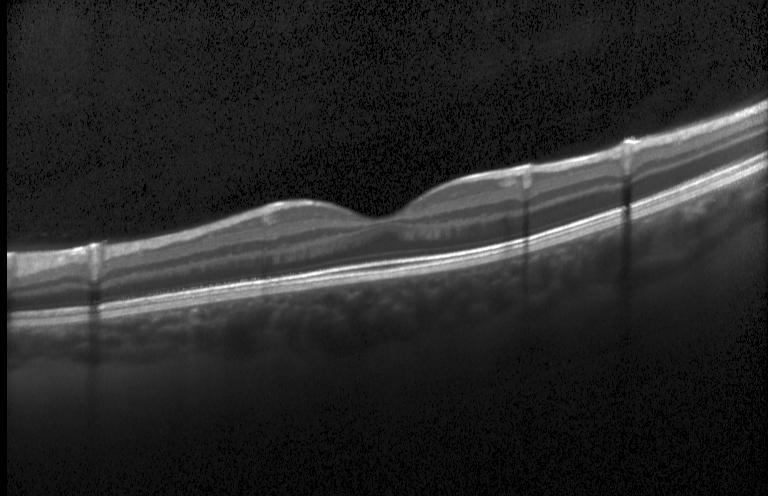 Optical coherence tomography B-scan; spectral-domain OCT — Neither choroidal neovascularization, diabetic macular edema, nor drusen.